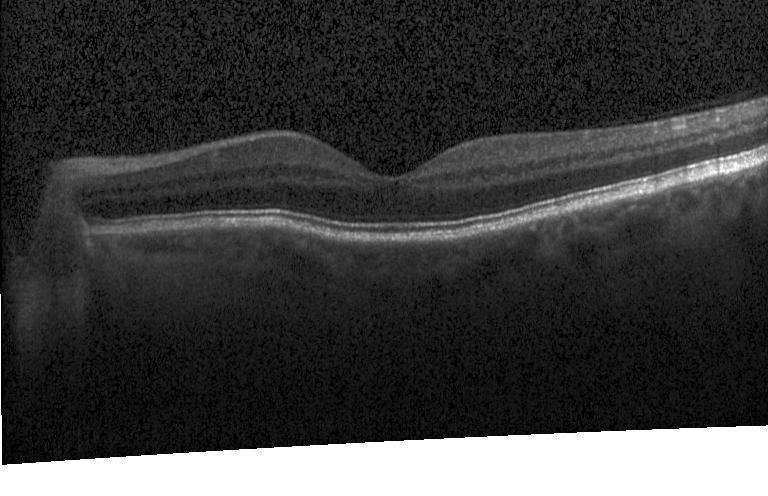 Optical coherence tomography scan
Dx: no choroidal neovascularization, no diabetic macular edema, and no drusen.